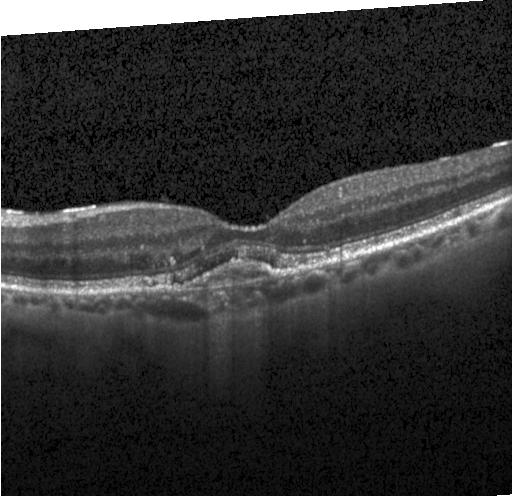

Finding: a choroidal neovascular membrane.